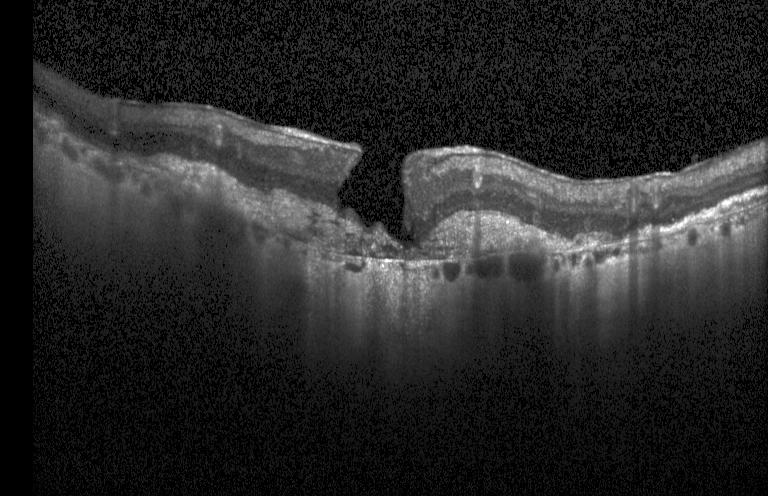 Heidelberg Spectralis; OCT B-scan. Impression: CNV.